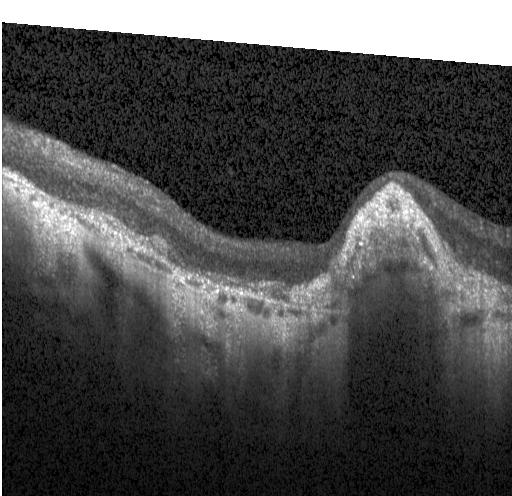

OCT scan showing a choroidal neovascular membrane.